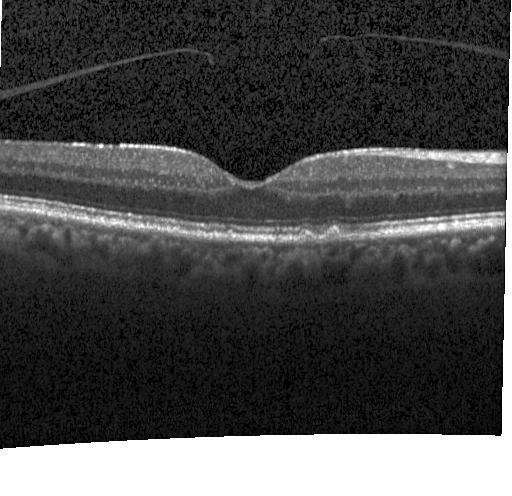
Finding: multiple drusen.